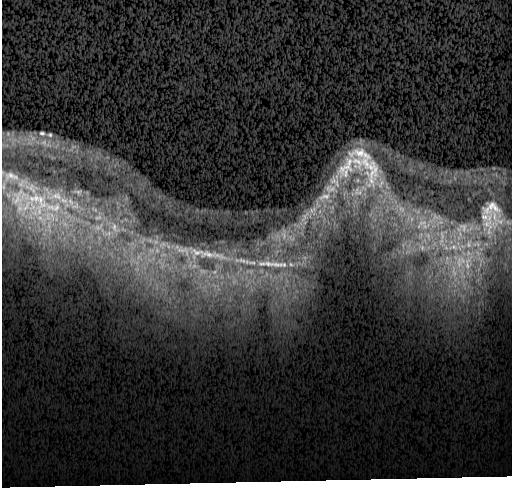

Horizontal scan through the fovea, acquired on a Heidelberg Spectralis, optical coherence tomography scan, spectral-domain optical coherence tomography — A choroidal neovascular membrane.